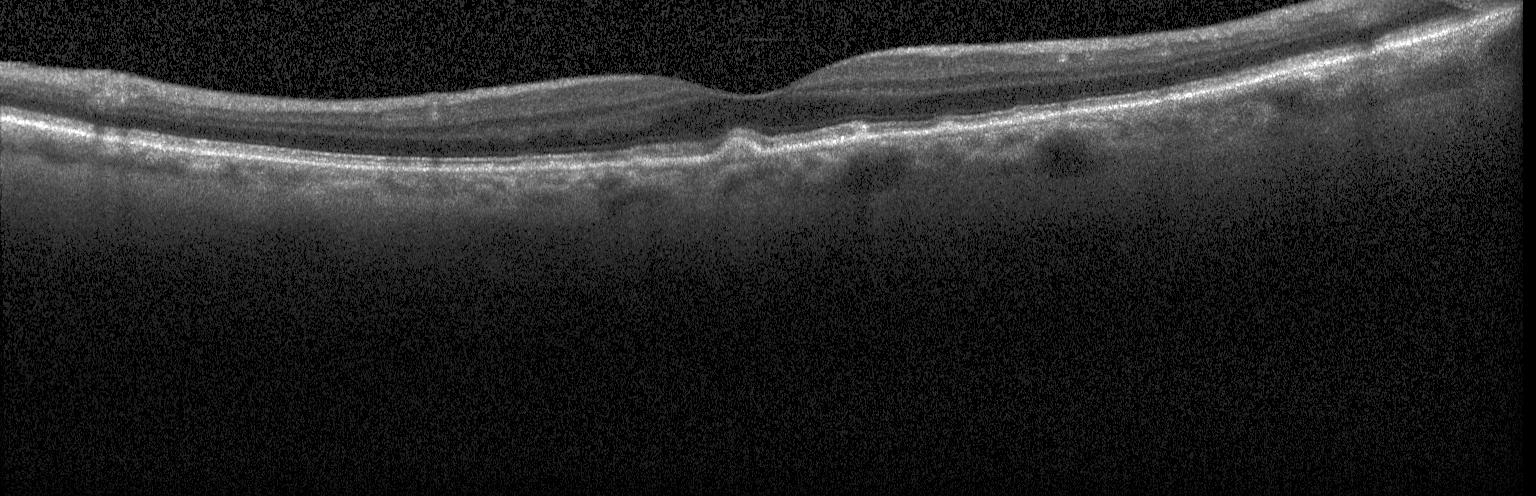
OCT finding: sub-RPE drusenoid deposits.